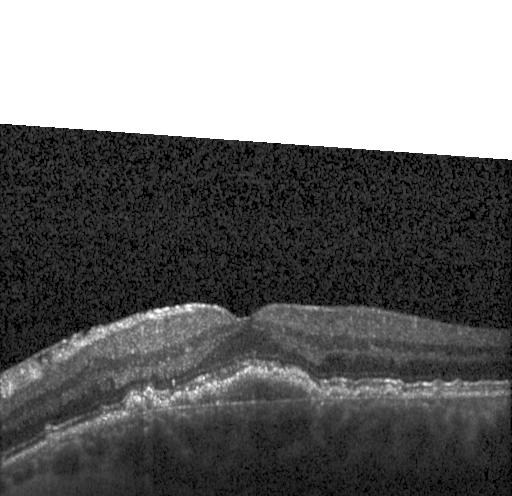
Macular OCT demonstrating choroidal neovascularization.